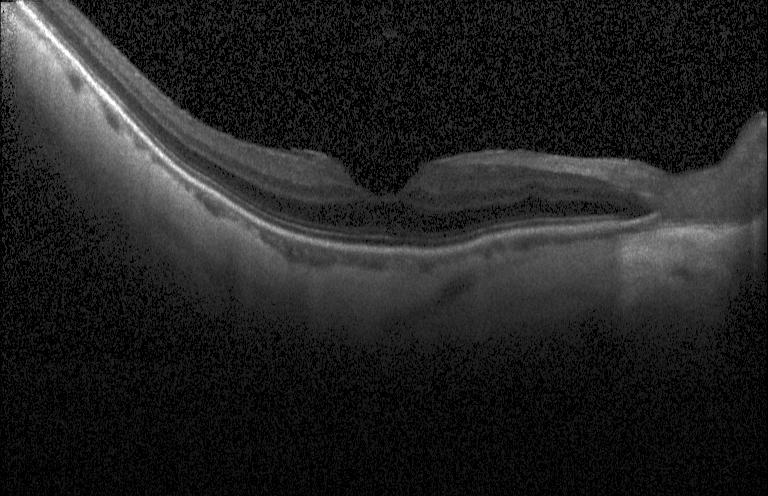
Retinal OCT B-scan.
This B-scan demonstrates no choroidal neovascularization, no diabetic macular edema, and no drusen.